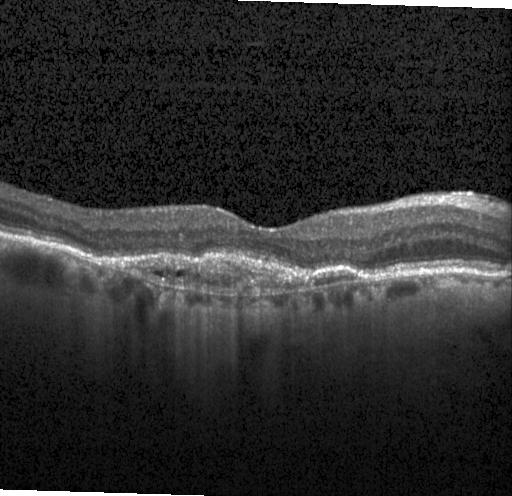

Retinal OCT cross-section.
The scan shows CNV.